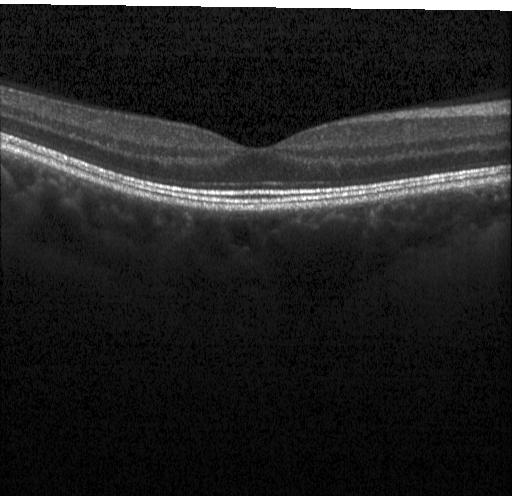
Diagnosis: neither choroidal neovascularization, diabetic macular edema, nor drusen.